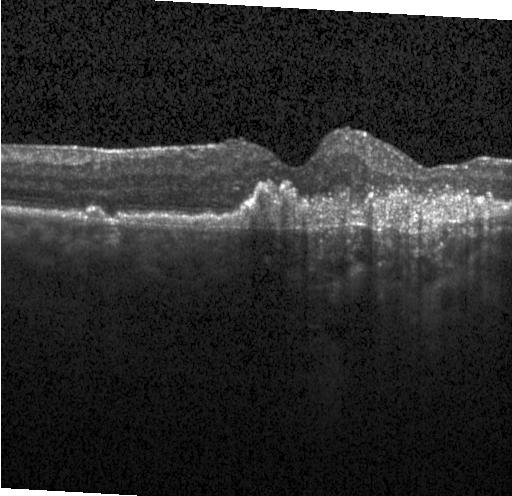

OCT B-scan — Diagnosis: choroidal neovascularization.